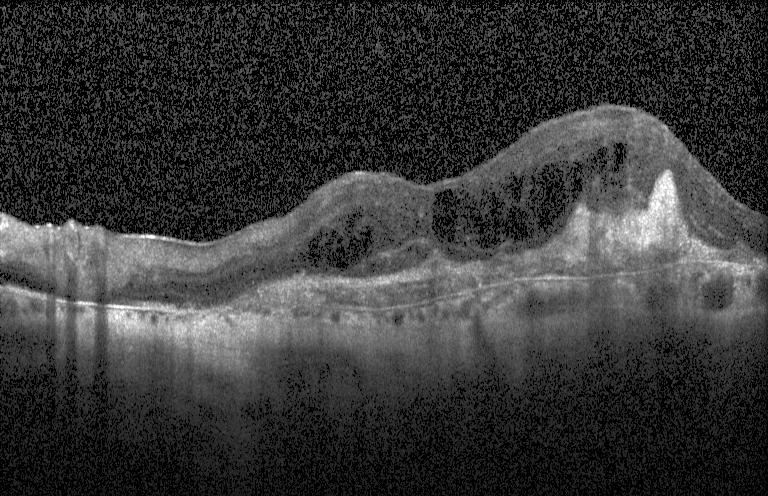

Optical coherence tomography scan. Diagnosis: a choroidal neovascular membrane.